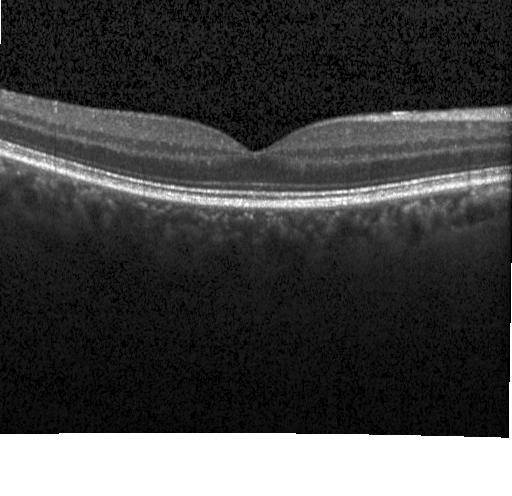
Retinal OCT cross-section showing no evidence of choroidal neovascularization, diabetic macular edema, or drusen.